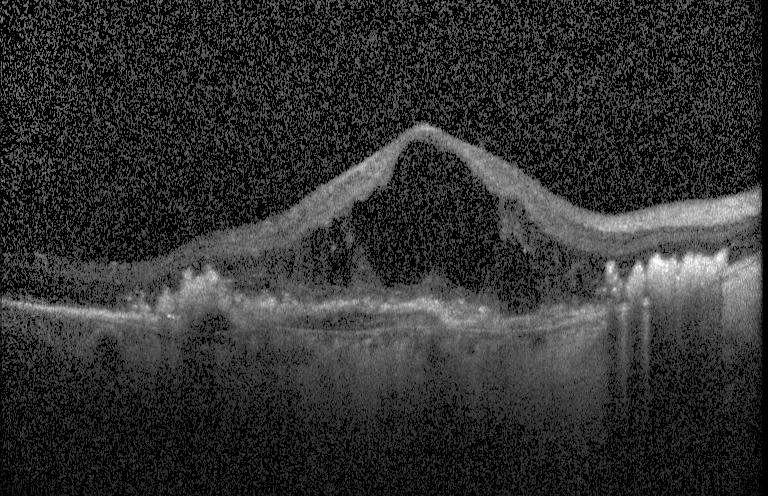
Retinal OCT cross-section · instrument: Heidelberg Spectralis · SD-OCT. Finding: a choroidal neovascular membrane.